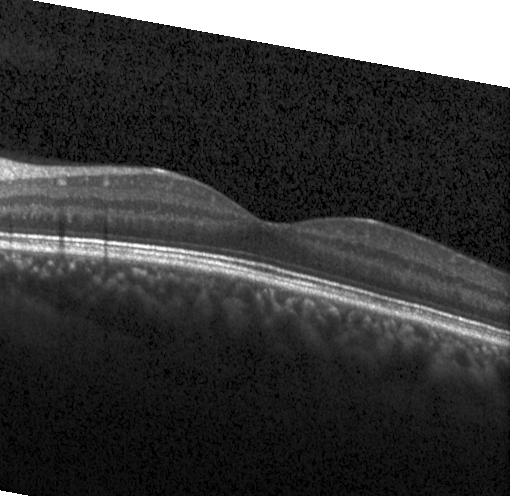 SD-OCT; Heidelberg Spectralis; through the macula; retinal OCT B-scan. Impression: no evidence of choroidal neovascularization, diabetic macular edema, or drusen.